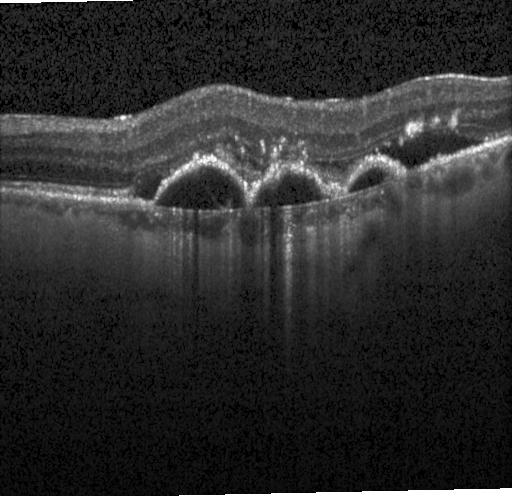
This B-scan demonstrates a choroidal neovascular membrane.